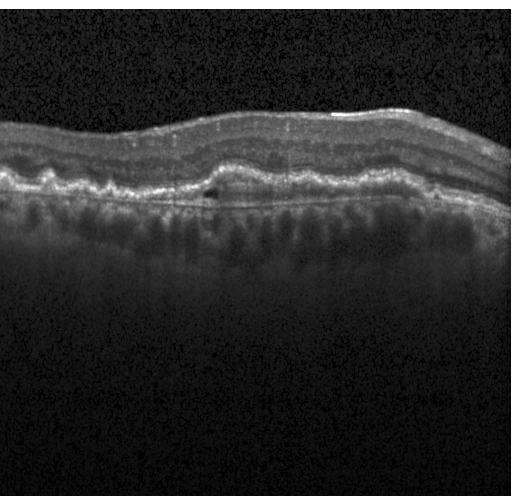

Centered on the fovea; OCT line scan. Diagnosis: a choroidal neovascular membrane.